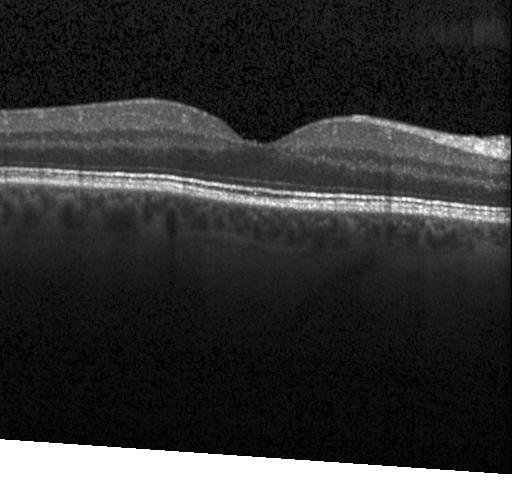
Retinal OCT B-scan · centered on the fovea · Heidelberg Spectralis · spectral-domain OCT — Impression: no evidence of CNV, DME, or drusen.